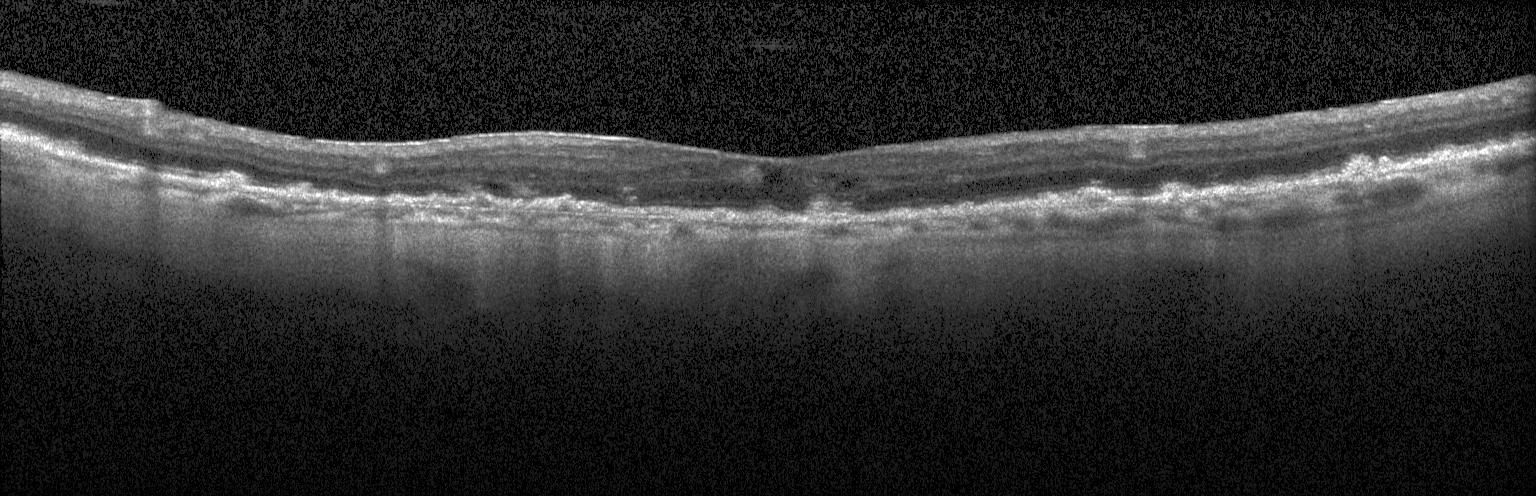
SD-OCT; Heidelberg Spectralis OCT system; centered on the fovea; OCT line scan. A choroidal neovascular membrane.